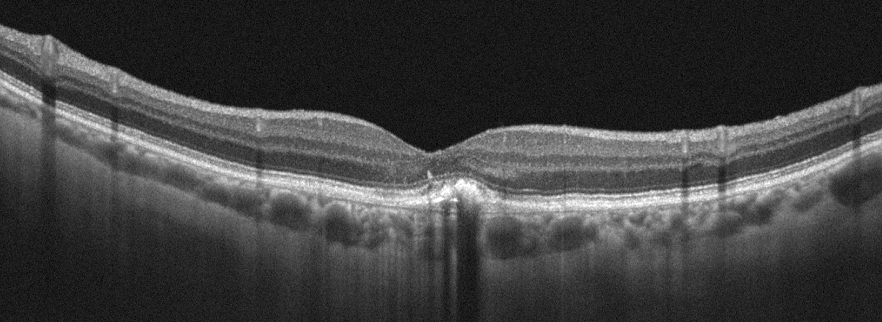
Macular OCT demonstrating AMD.